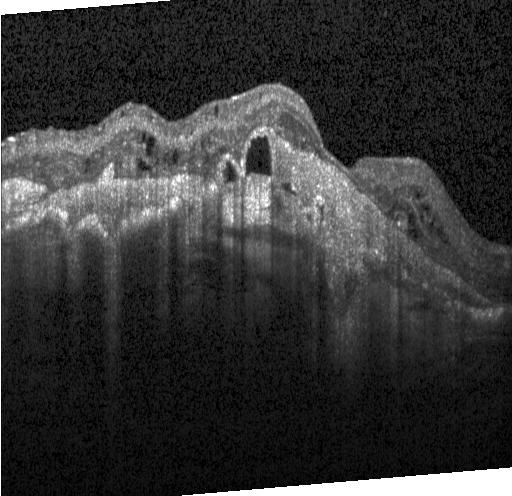

OCT finding: a choroidal neovascular membrane.